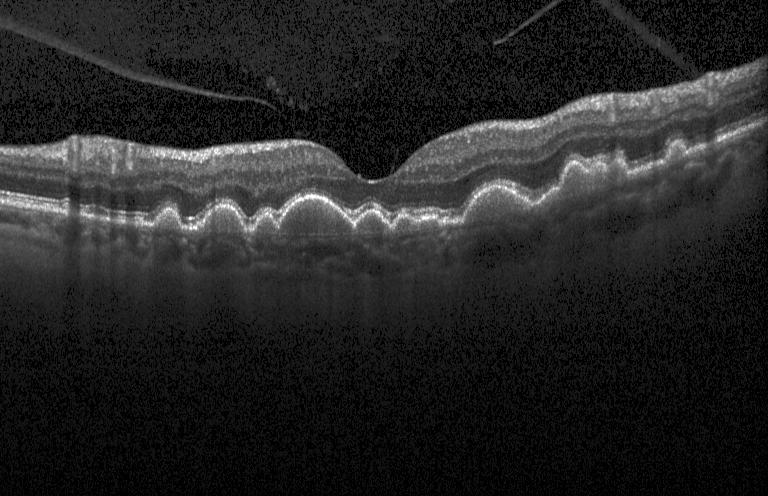
Acquired on a Heidelberg Spectralis, retinal OCT B-scan, spectral-domain OCT, through the macula. Finding: sub-RPE drusenoid deposits.